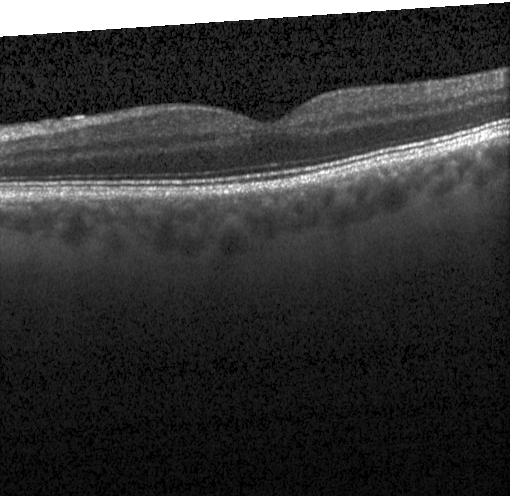
Acquired on a Heidelberg Spectralis; fovea-centered; spectral-domain optical coherence tomography; OCT B-scan.
Impression: no evidence of choroidal neovascularization, diabetic macular edema, or drusen.